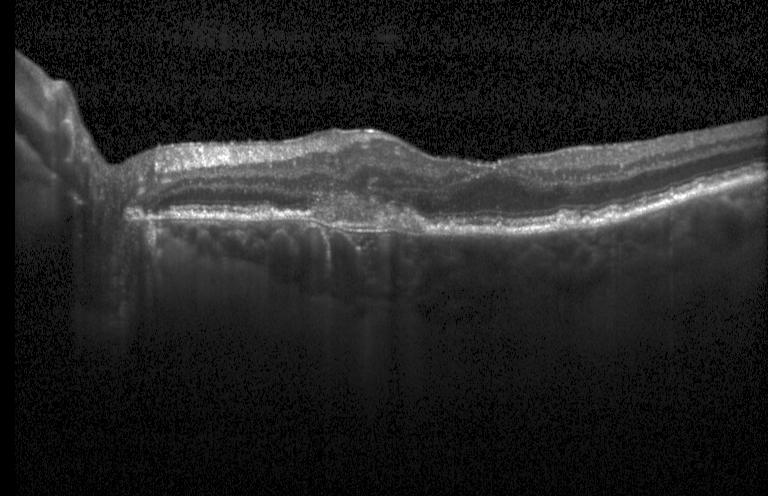
Optical coherence tomography B-scan · SD-OCT · horizontal scan through the fovea · Heidelberg Spectralis OCT system
Impression: a choroidal neovascular membrane.